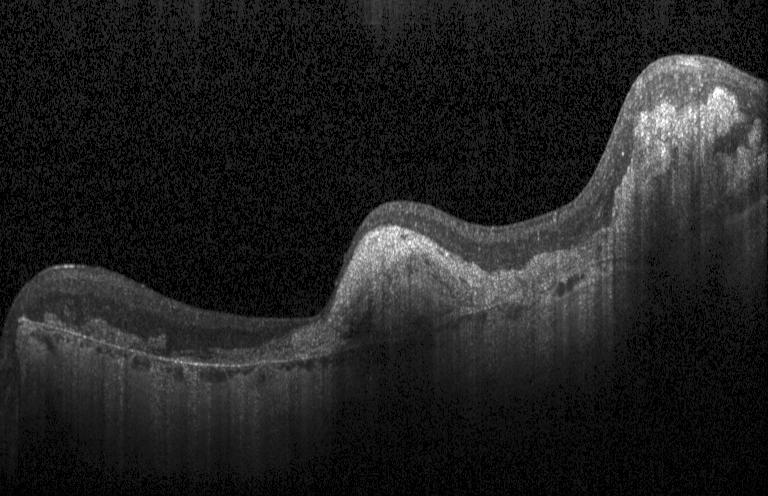

Spectral-domain OCT B-scan: a choroidal neovascular membrane.